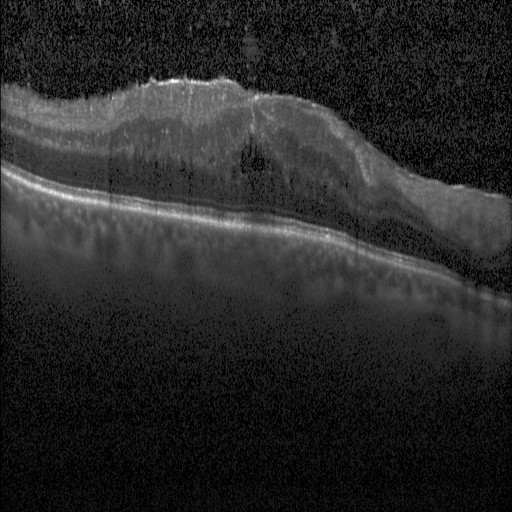

Retinal OCT cross-section. Spectral-domain OCT.
This B-scan demonstrates DME.